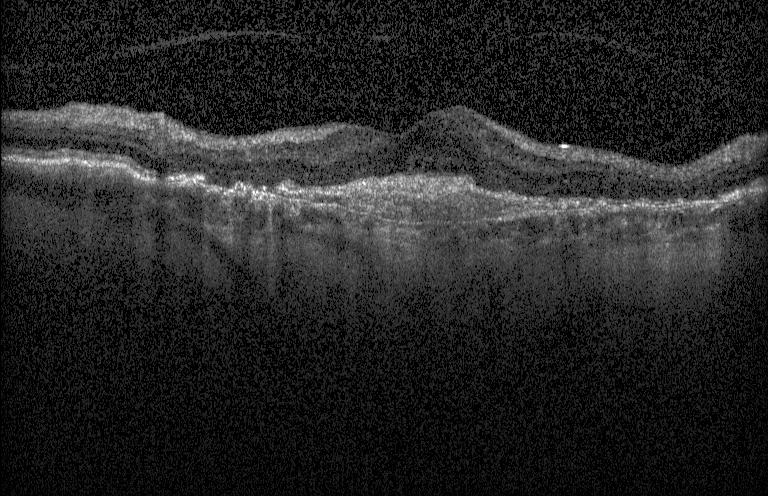
Optical coherence tomography B-scan
The scan shows a choroidal neovascular membrane.